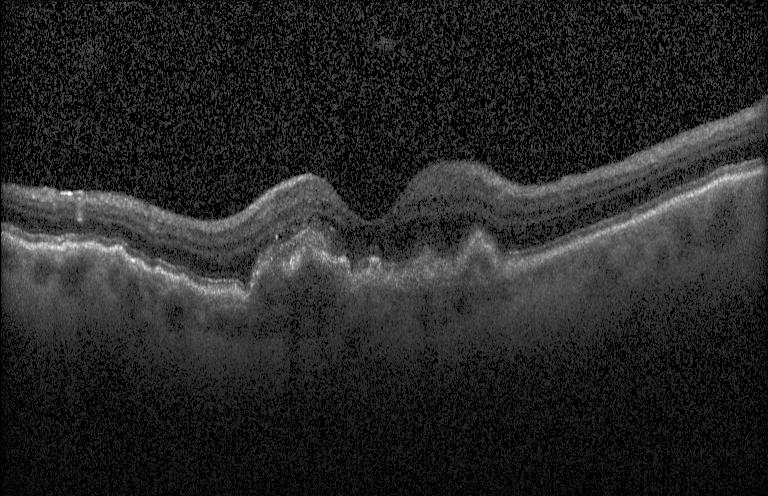
Heidelberg Spectralis. Centered on the fovea. OCT B-scan — Diagnosis: a choroidal neovascular membrane.